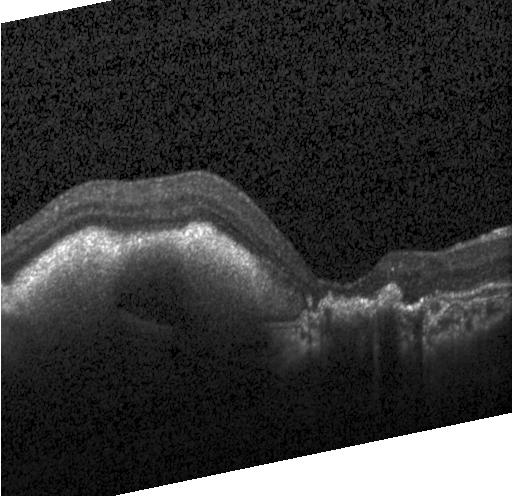 Finding: a choroidal neovascular membrane.